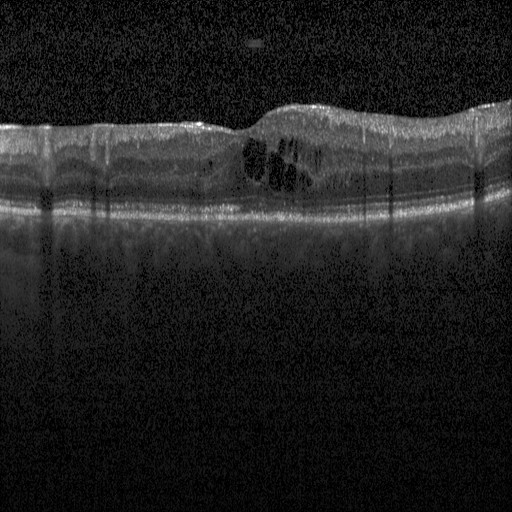

Instrument: Heidelberg Spectralis. Optical coherence tomography scan
This B-scan demonstrates diabetic macular edema (DME).